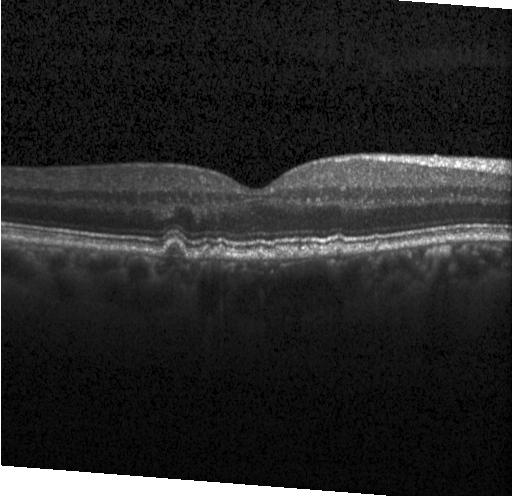
Retinal OCT B-scan · SD-OCT · Heidelberg Spectralis OCT system · macular scan.
Diagnosis: multiple drusen.